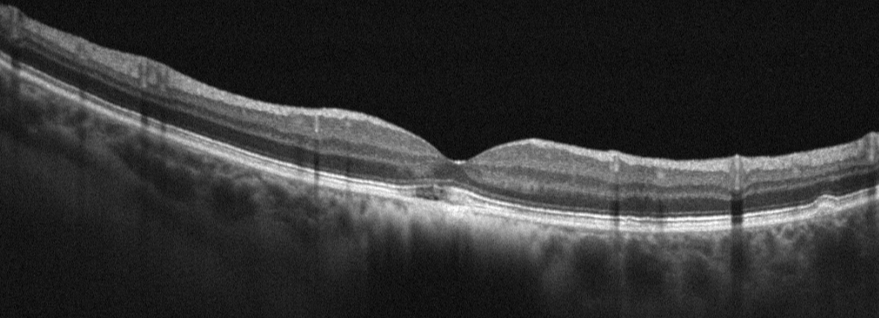

Assessment: age-related macular degeneration.